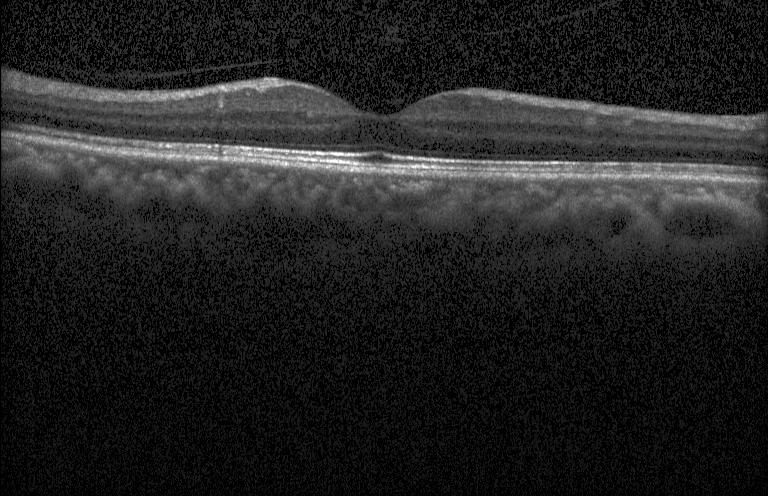
Macular OCT demonstrating no evidence of choroidal neovascularization, diabetic macular edema, or drusen.